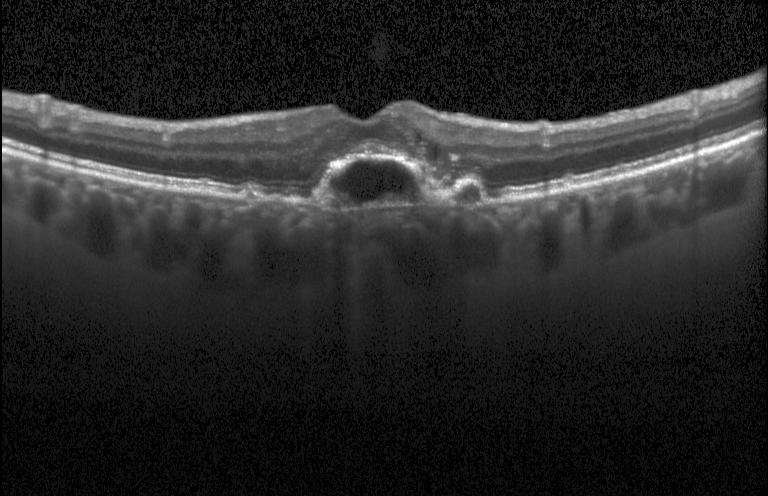
Optical coherence tomography B-scan
Dx: a choroidal neovascular membrane.